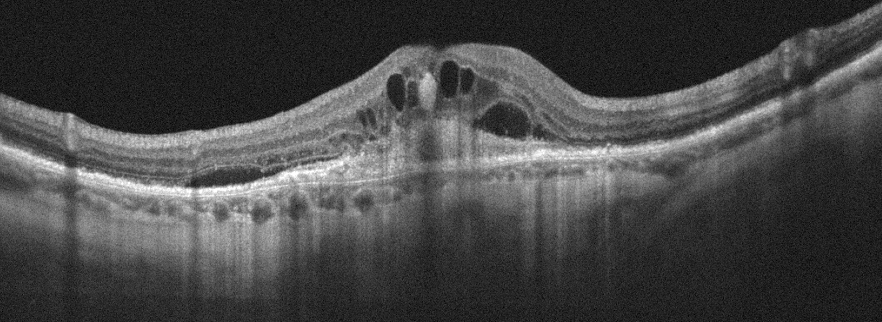
Diagnosis: AMD.